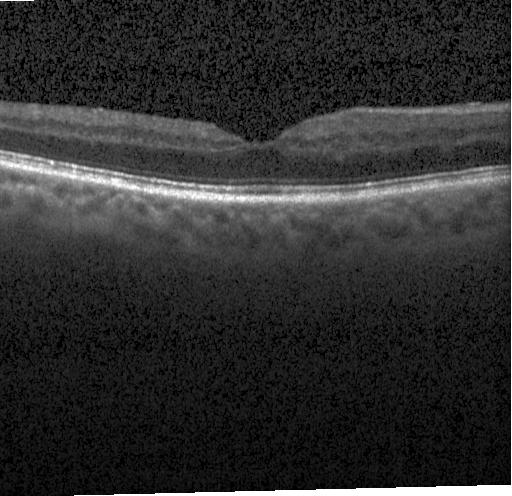
Optical coherence tomography scan. This B-scan demonstrates no CNV, no DME, and no drusen.